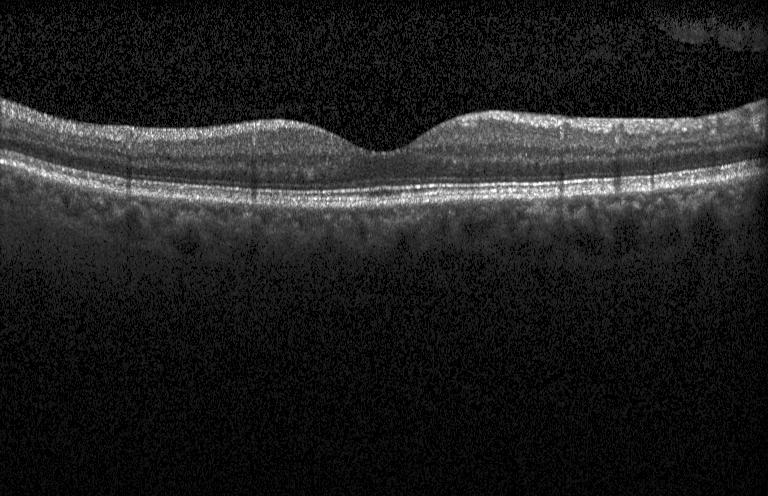

Optical coherence tomography scan. This B-scan demonstrates no choroidal neovascularization, diabetic macular edema, or drusen.